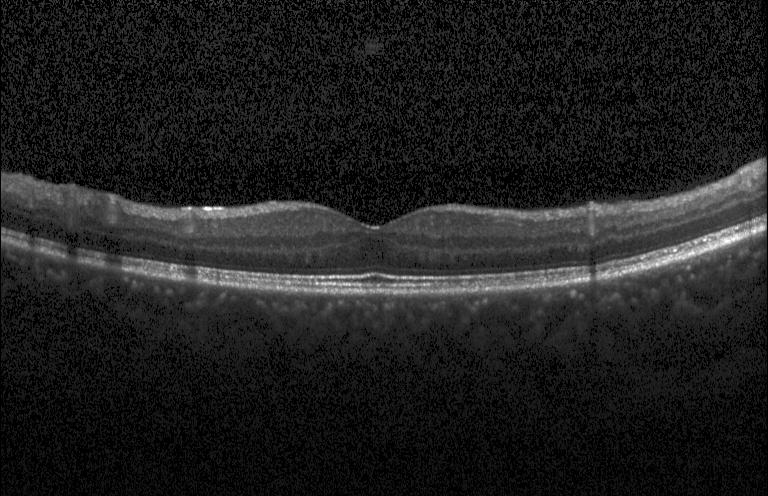
Retinal OCT B-scan
No CNV, DME, or drusen.